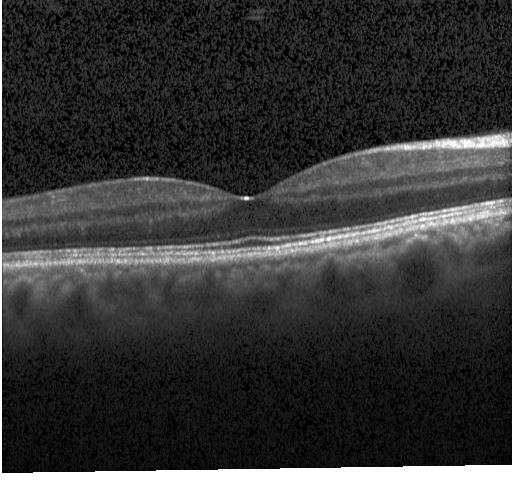 Spectral-domain OCT, OCT line scan, centered on the fovea.
Assessment: no choroidal neovascularization, diabetic macular edema, or drusen.